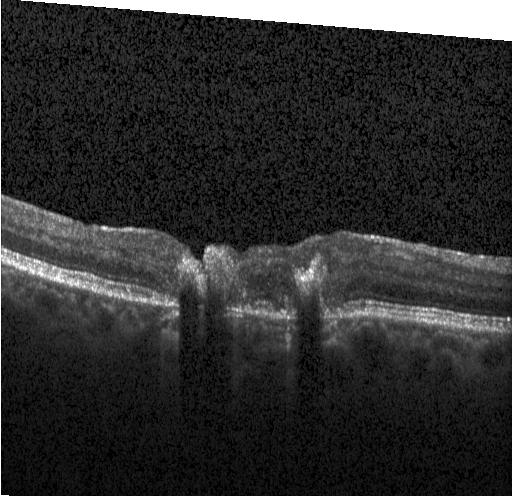
Macular scan. Heidelberg Spectralis. Spectral-domain OCT. Optical coherence tomography scan.
This B-scan demonstrates choroidal neovascularization.